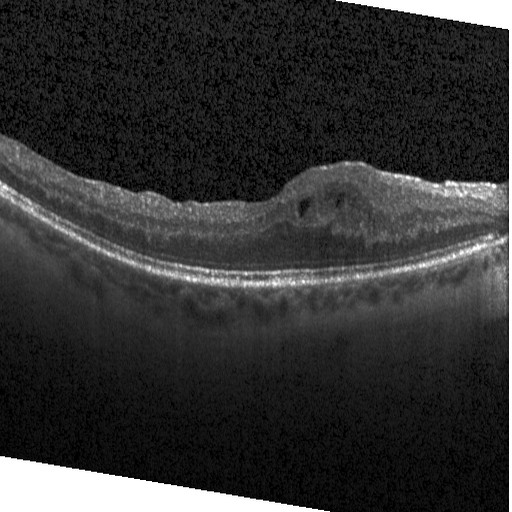

Retinal OCT cross-section. The scan shows DME.